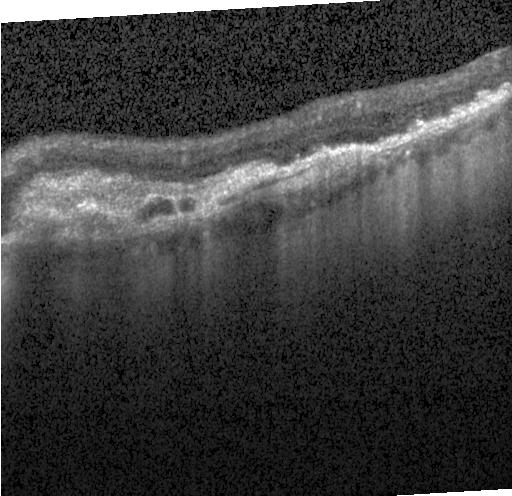
Spectral-domain optical coherence tomography · Heidelberg Spectralis OCT system · retinal OCT B-scan.
Finding: choroidal neovascularization (CNV).